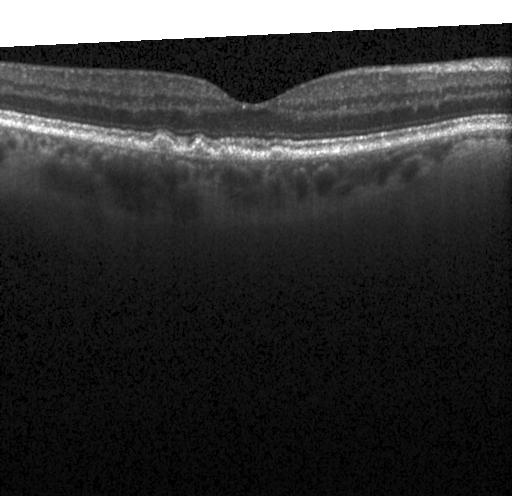
OCT finding: drusen.